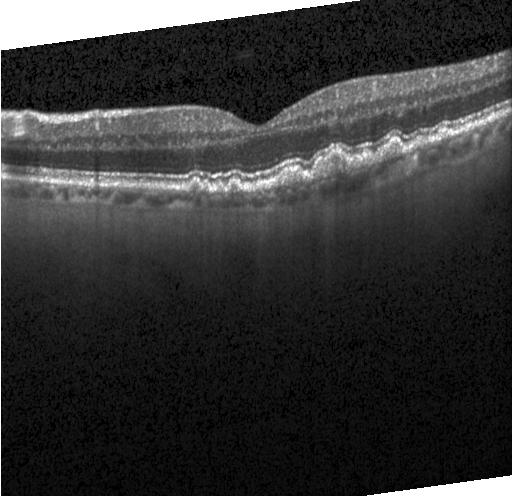

OCT line scan — OCT finding: multiple drusen.